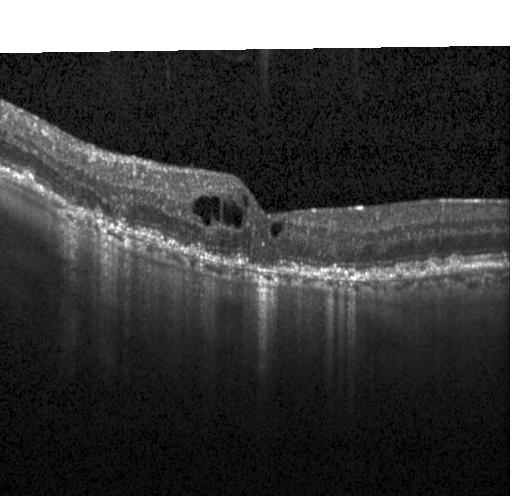 Diagnosis: choroidal neovascularization.